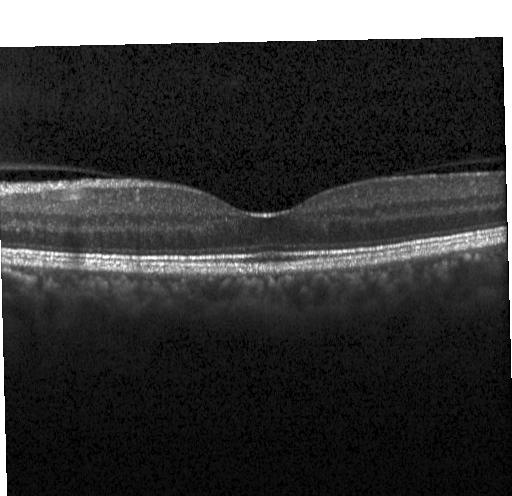
OCT line scan. Heidelberg Spectralis — Diagnosis: neither choroidal neovascularization, diabetic macular edema, nor drusen.